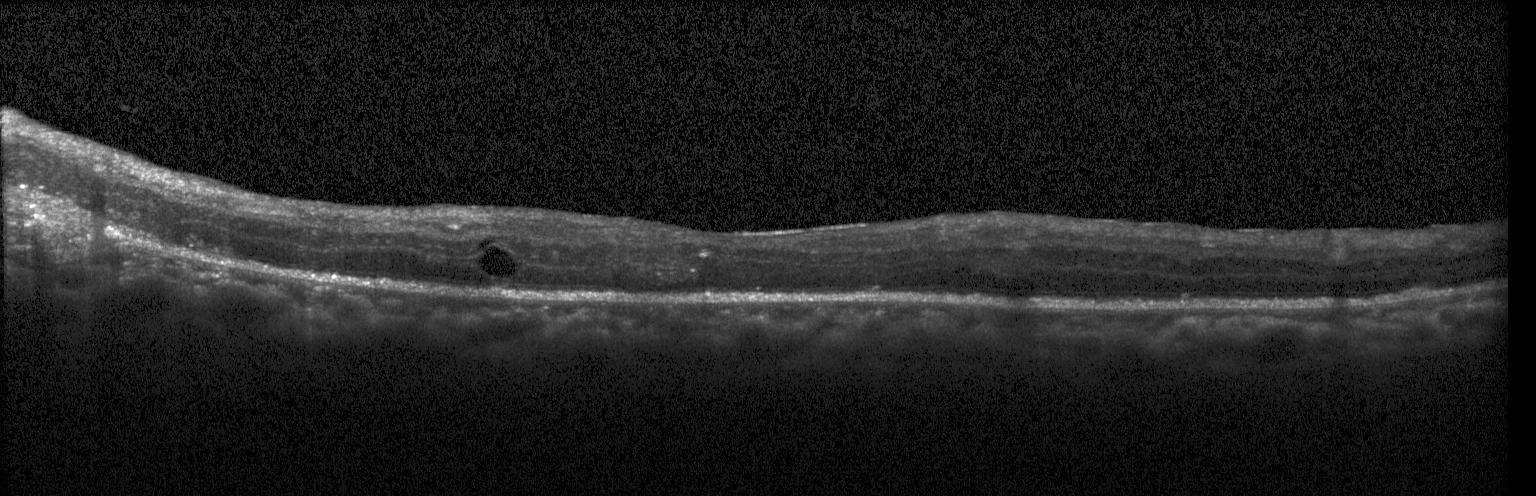 Optical coherence tomography B-scan · macular scan · spectral-domain OCT. OCT finding: diabetic macular edema (DME).